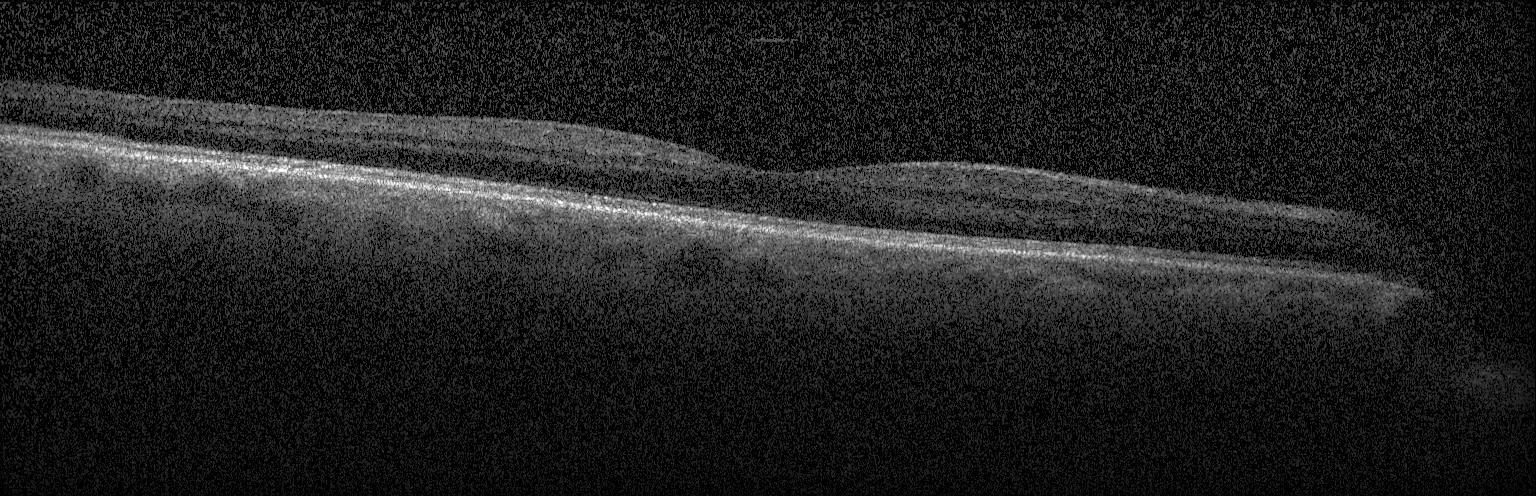
No evidence of choroidal neovascularization, diabetic macular edema, or drusen.